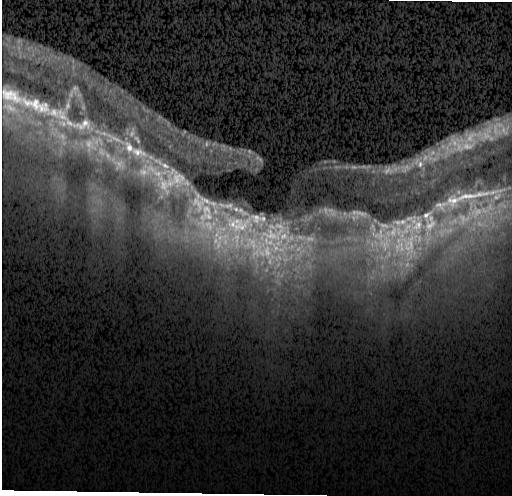 Impression: CNV.